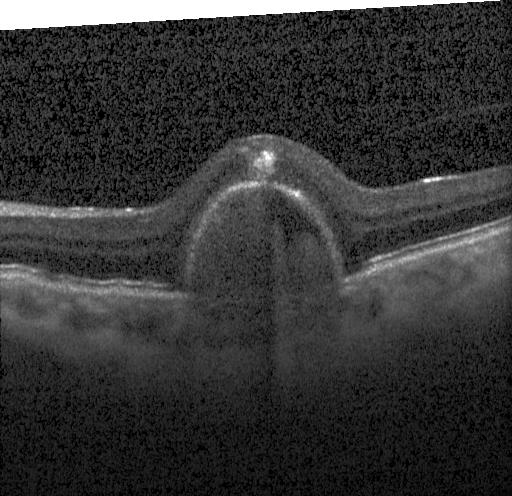
Macular OCT: a choroidal neovascular membrane.